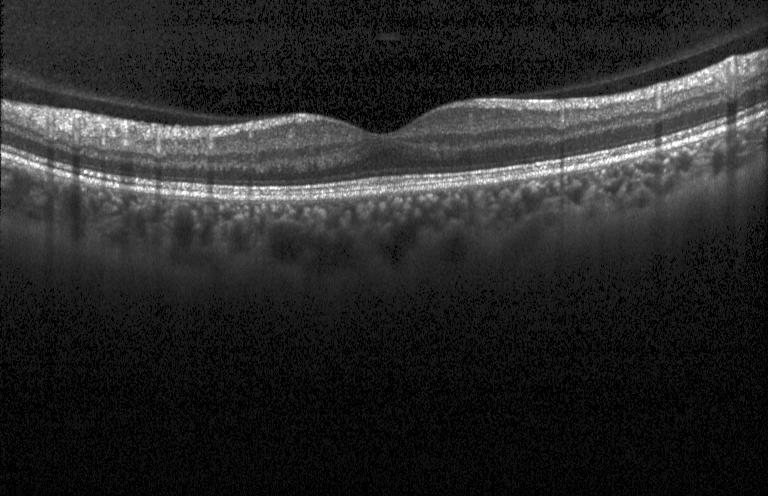 Spectral-domain optical coherence tomography. Acquired on a Heidelberg Spectralis. Retinal OCT cross-section
No choroidal neovascularization, no diabetic macular edema, and no drusen.